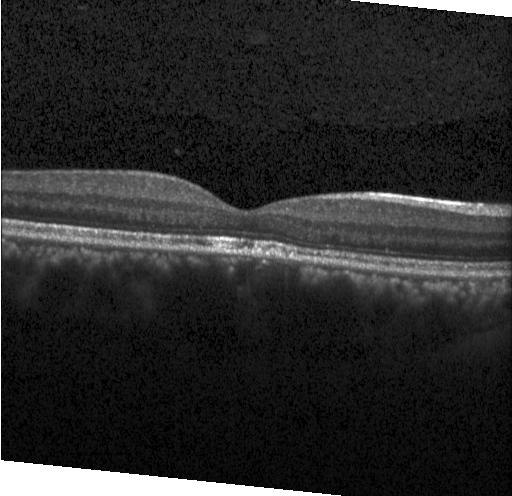

Optical coherence tomography scan.
No evidence of choroidal neovascularization, diabetic macular edema, or drusen.